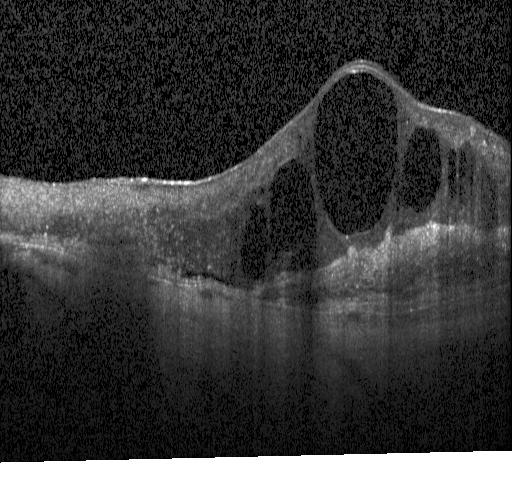
Optical coherence tomography B-scan
Finding: a choroidal neovascular membrane.